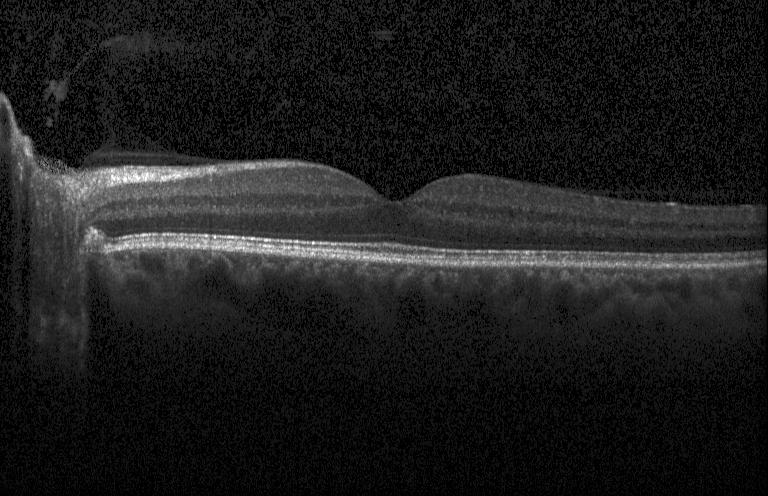
Optical coherence tomography scan.
Finding: no choroidal neovascularization, no diabetic macular edema, and no drusen.